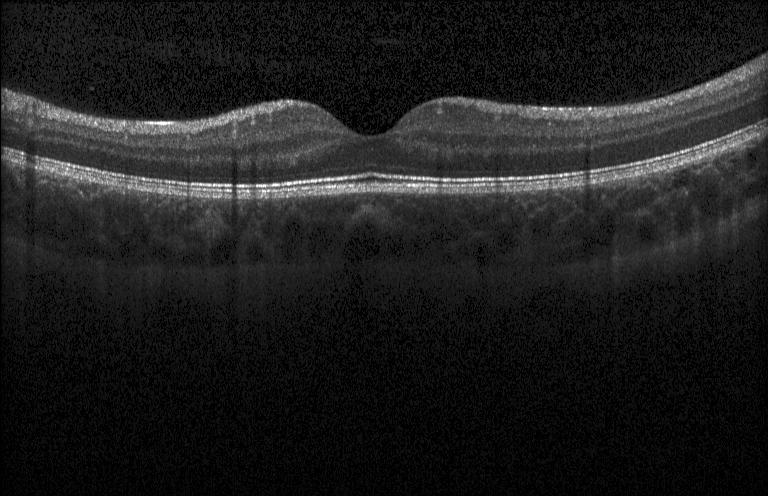 Optical coherence tomography scan, horizontal scan through the fovea, spectral-domain OCT
Neither choroidal neovascularization, diabetic macular edema, nor drusen.